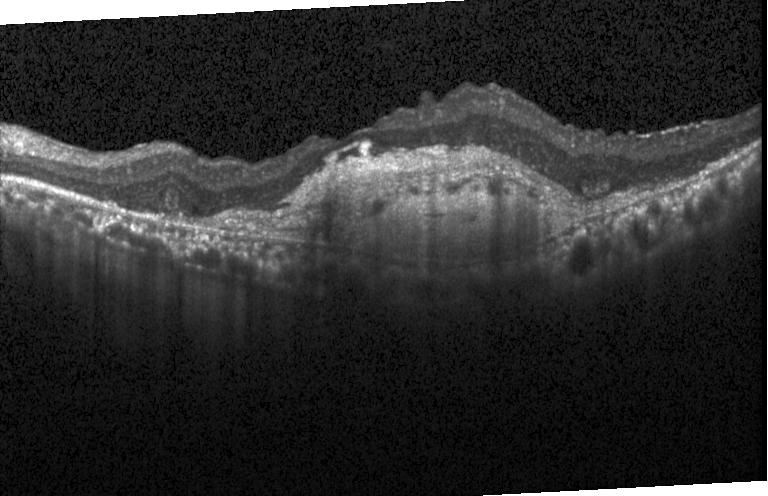
Optical coherence tomography B-scan, through the macula.
Assessment: a choroidal neovascular membrane.